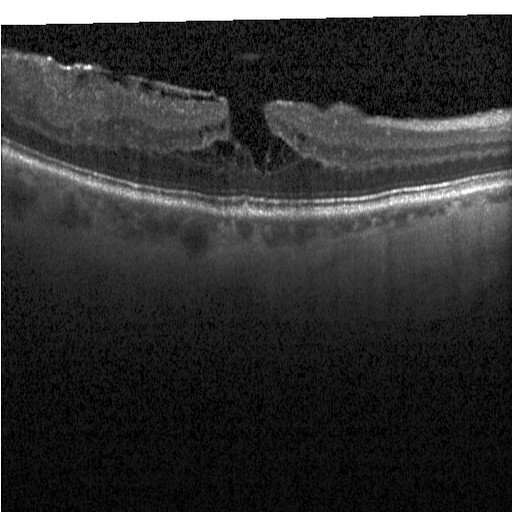
OCT B-scan.
Diagnosis: diabetic macular edema.